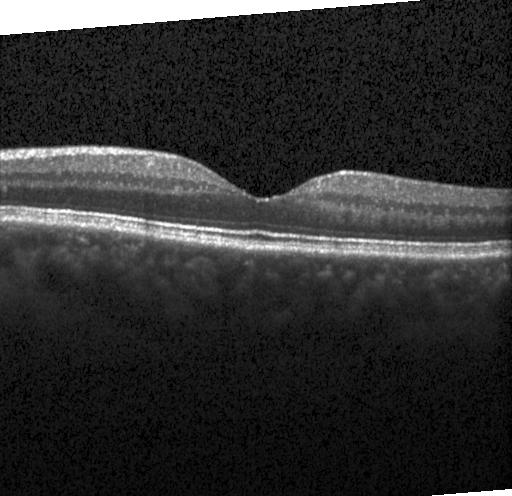 Diagnosis: no evidence of choroidal neovascularization, diabetic macular edema, or drusen.